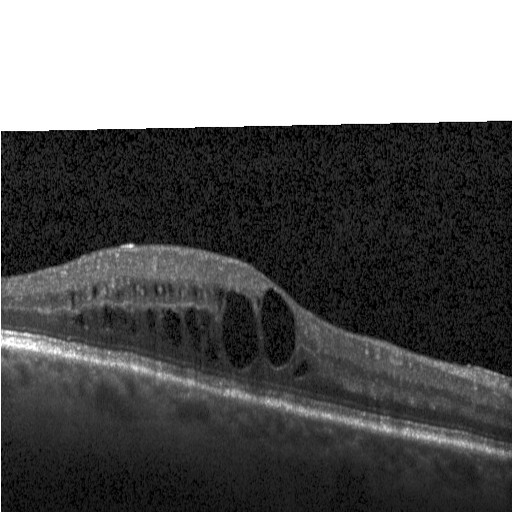 OCT finding: diabetic macular edema.